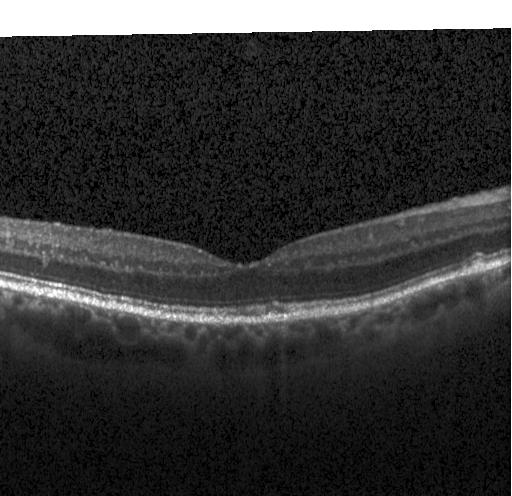 OCT scan showing drusen.